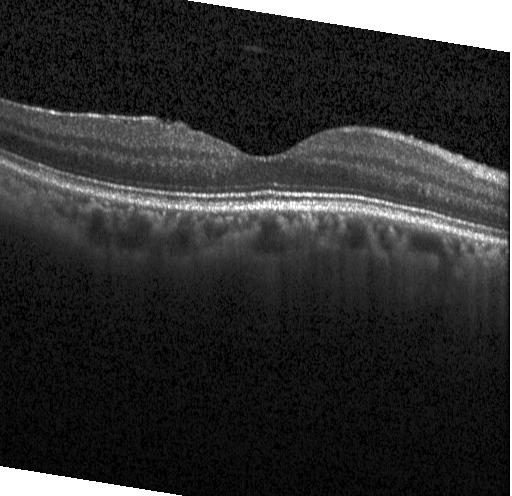
OCT B-scan. Impression: no CNV, DME, or drusen.